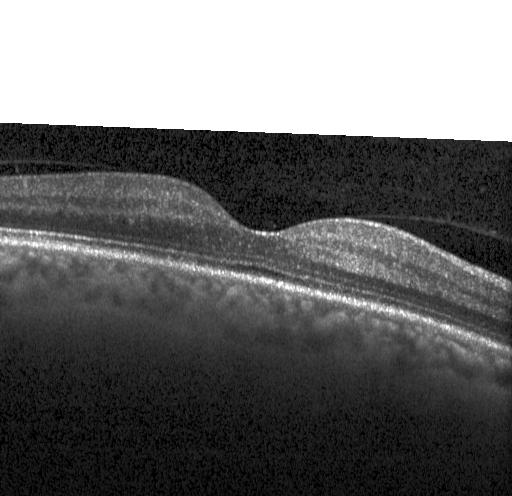

Retinal OCT cross-section · instrument: Heidelberg Spectralis
Finding: no CNV, no DME, and no drusen.